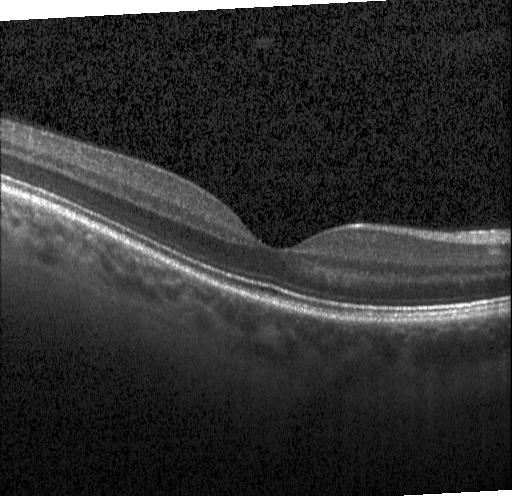
Retinal OCT cross-section — Diagnosis: no choroidal neovascularization, no diabetic macular edema, and no drusen.